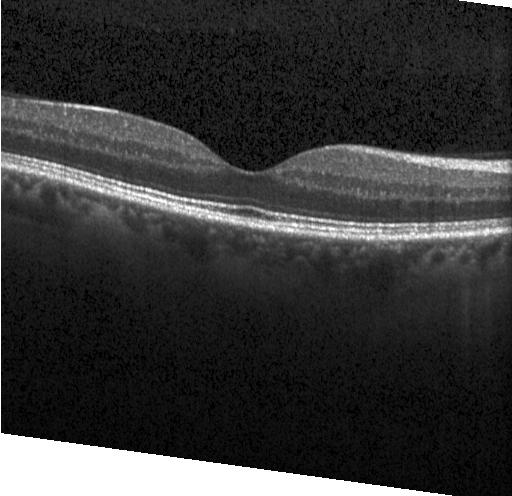 OCT B-scan showing no choroidal neovascularization, diabetic macular edema, or drusen.